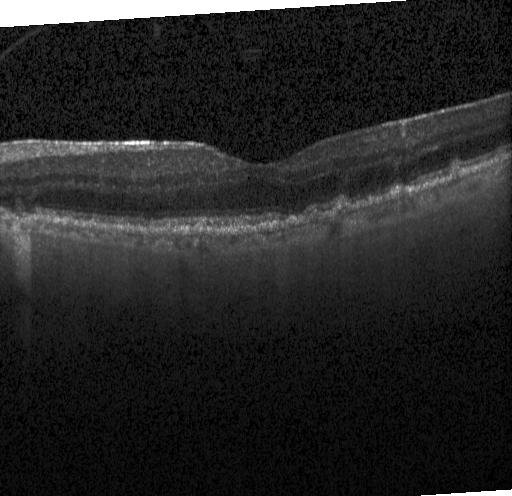 Retinal OCT B-scan, centered on the fovea, acquired on a Heidelberg Spectralis. Diagnosis: sub-RPE drusenoid deposits.